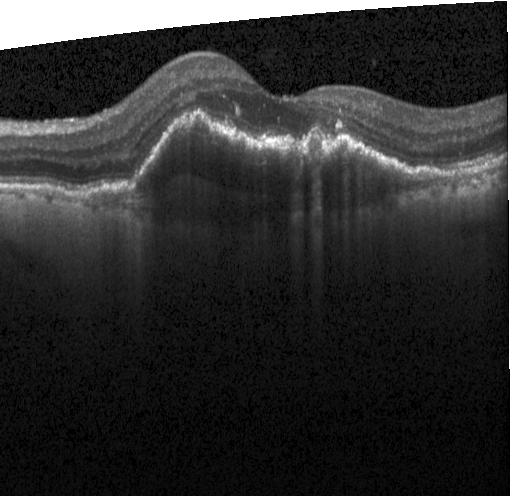
Finding: a choroidal neovascular membrane.